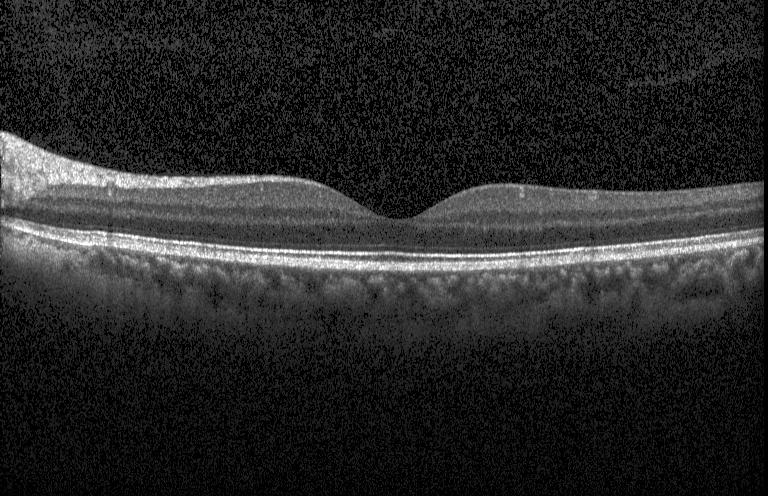 Macular OCT demonstrating no CNV, DME, or drusen.